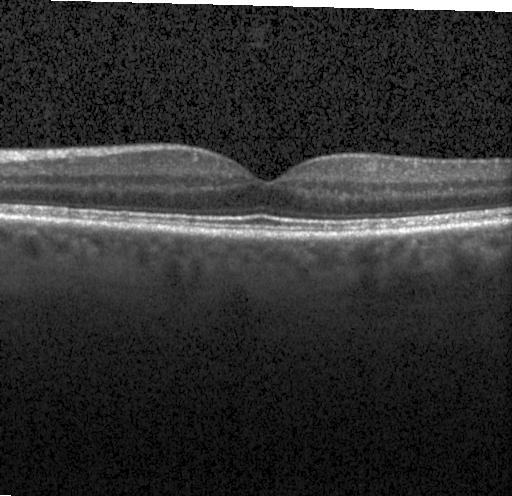 Dx: neither choroidal neovascularization, diabetic macular edema, nor drusen.